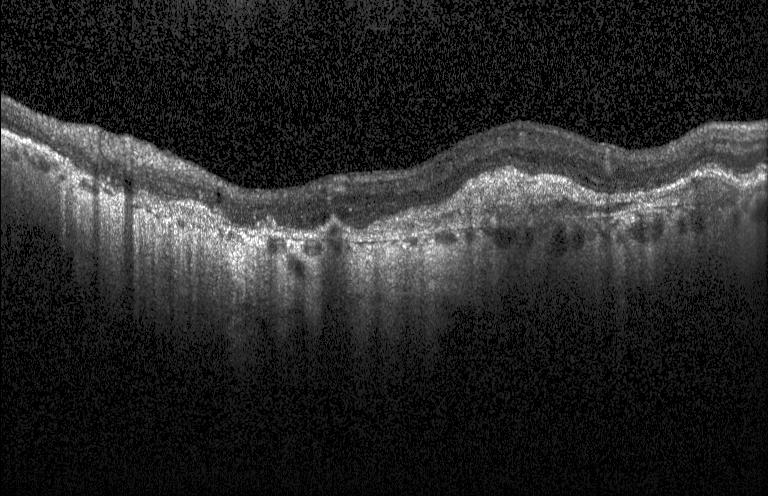

Retinal OCT cross-section, spectral-domain optical coherence tomography — Macular OCT: choroidal neovascularization.